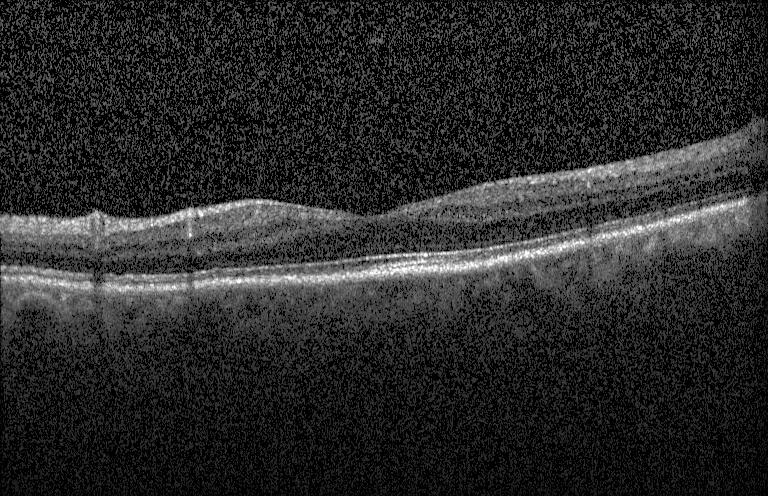

Retinal OCT cross-section; Heidelberg Spectralis; through the macula
Diagnosis: no evidence of choroidal neovascularization, diabetic macular edema, or drusen.